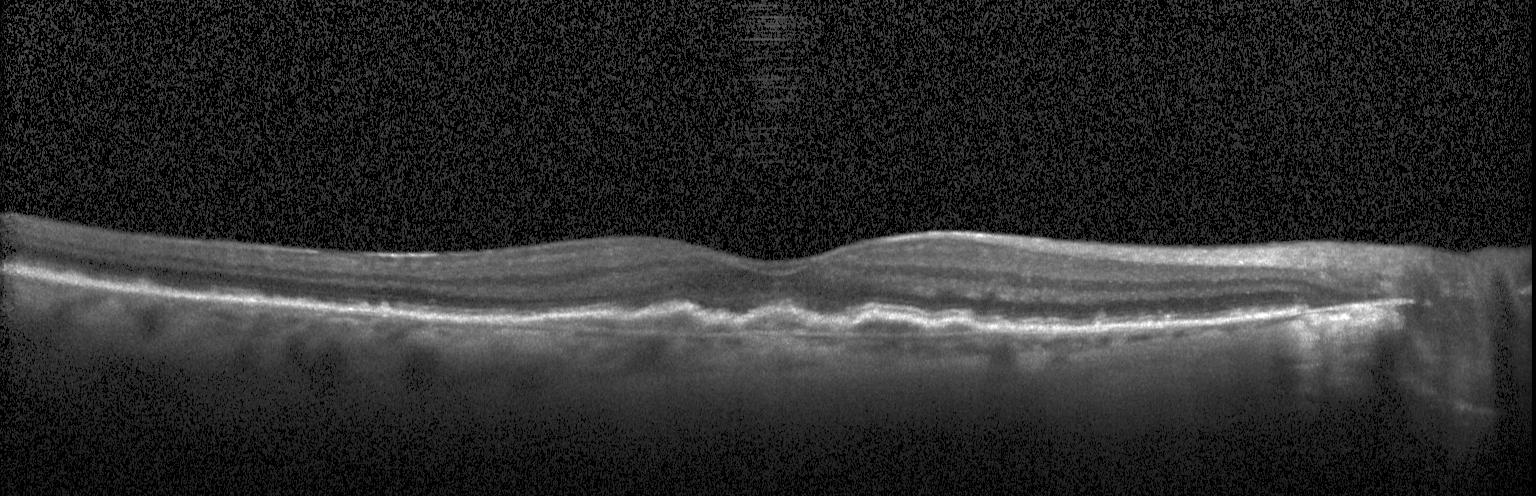
SD-OCT · OCT B-scan.
Impression: choroidal neovascularization.